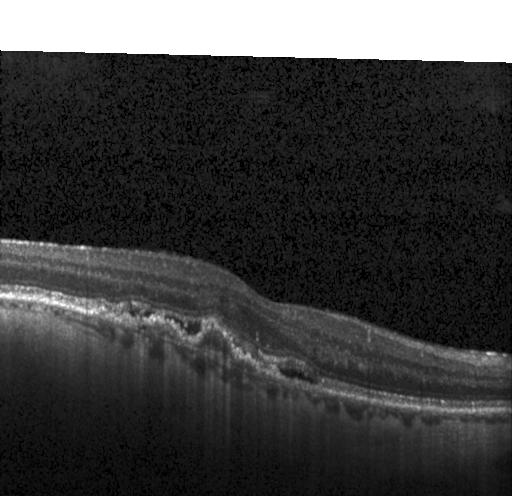
SD-OCT; fovea-centered; optical coherence tomography scan; Heidelberg Spectralis OCT system.
A choroidal neovascular membrane.